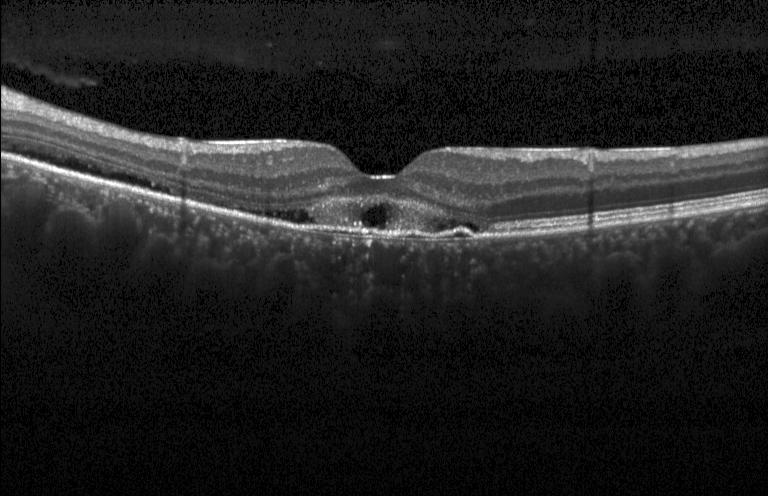 Assessment: a choroidal neovascular membrane.